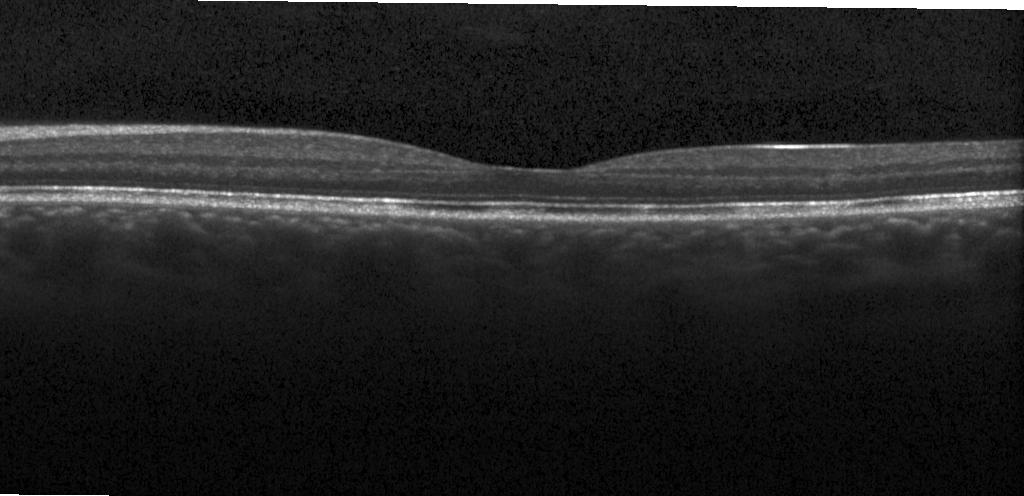 SD-OCT; Heidelberg Spectralis OCT system; through the macula; OCT B-scan — Impression: no CNV, DME, or drusen.